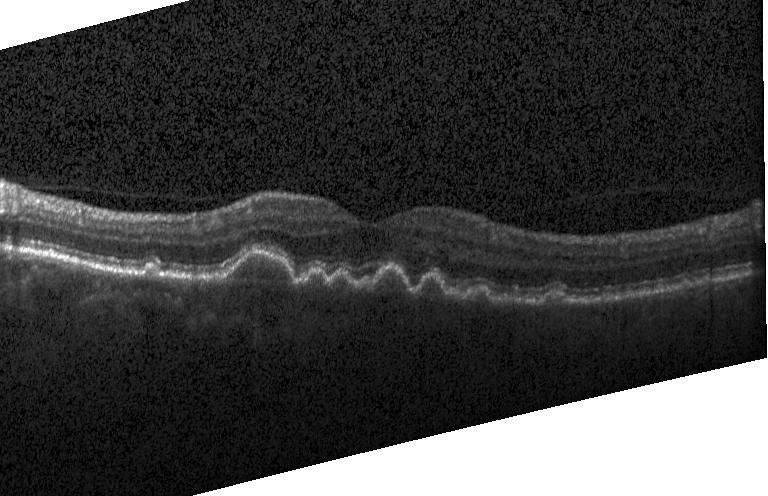
Retinal OCT cross-section showing sub-RPE drusenoid deposits.